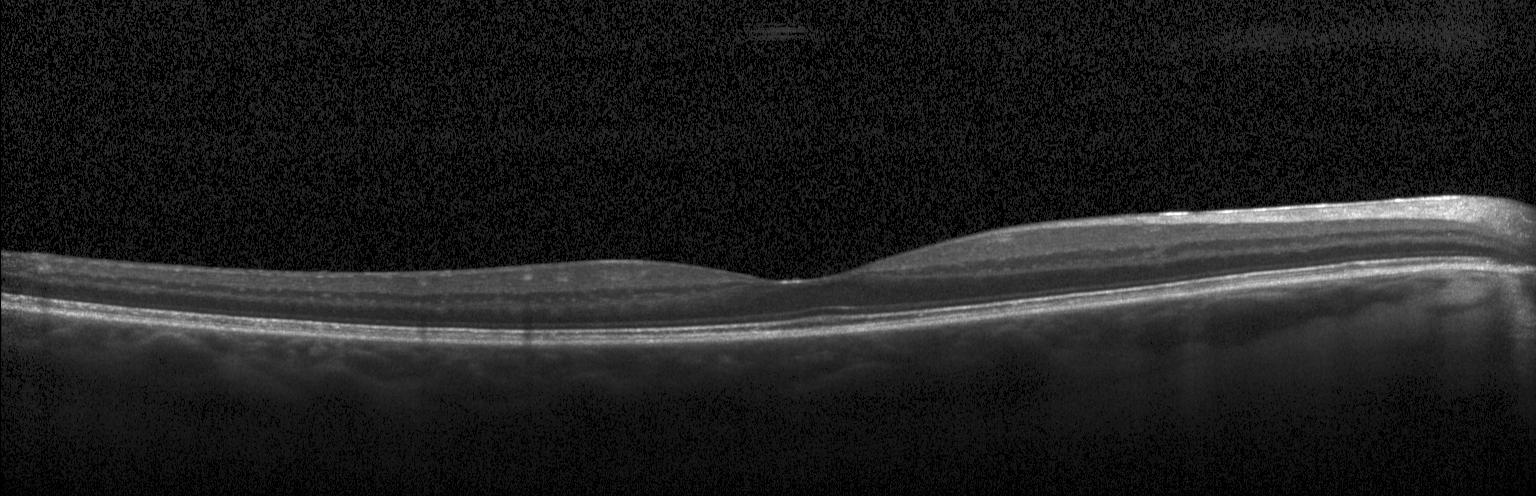

Diagnosis: no evidence of choroidal neovascularization, diabetic macular edema, or drusen.